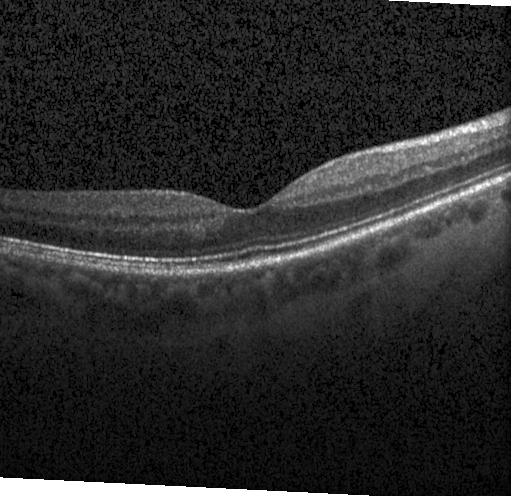 OCT B-scan. Instrument: Heidelberg Spectralis. Macular scan. Spectral-domain optical coherence tomography.
The scan shows no choroidal neovascularization, diabetic macular edema, or drusen.